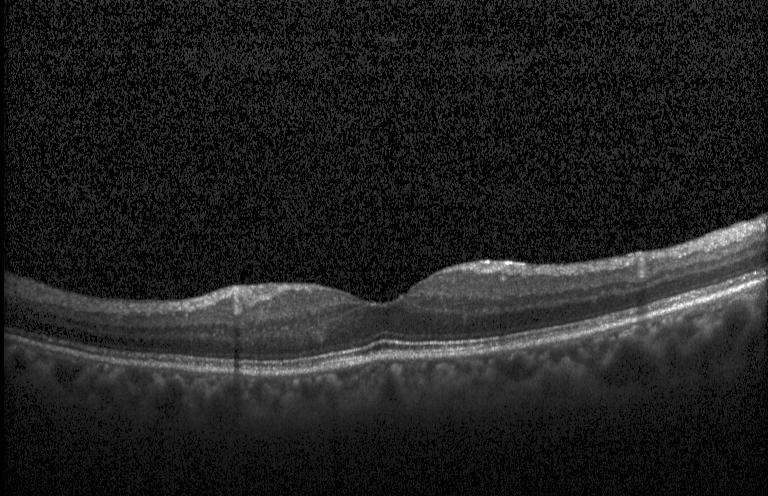

OCT B-scan showing no choroidal neovascularization, no diabetic macular edema, and no drusen.